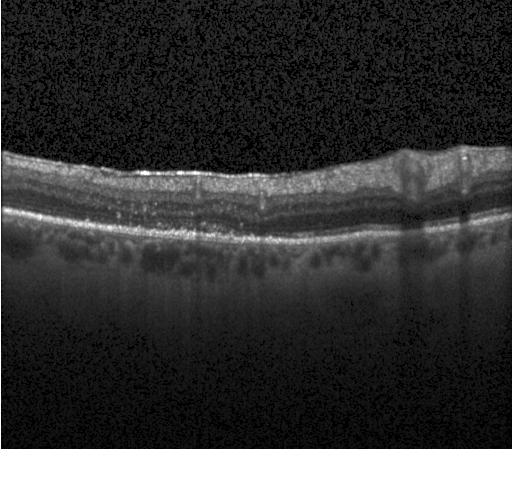

Macular scan, Heidelberg Spectralis, retinal OCT B-scan. Impression: a choroidal neovascular membrane.